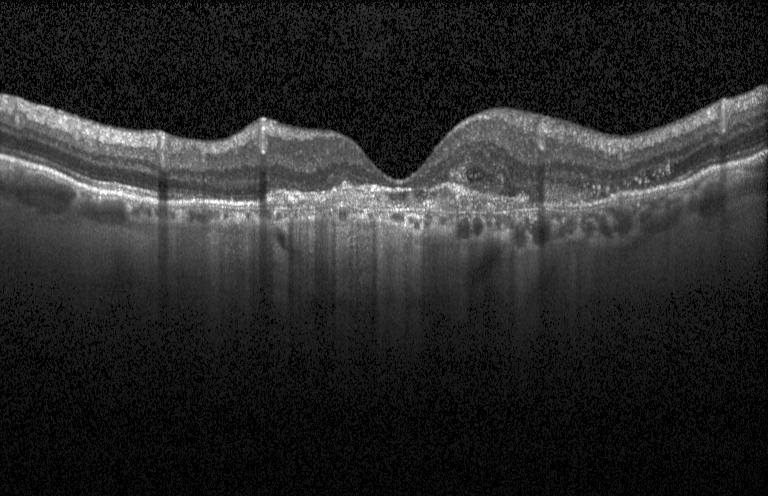

Choroidal neovascularization.